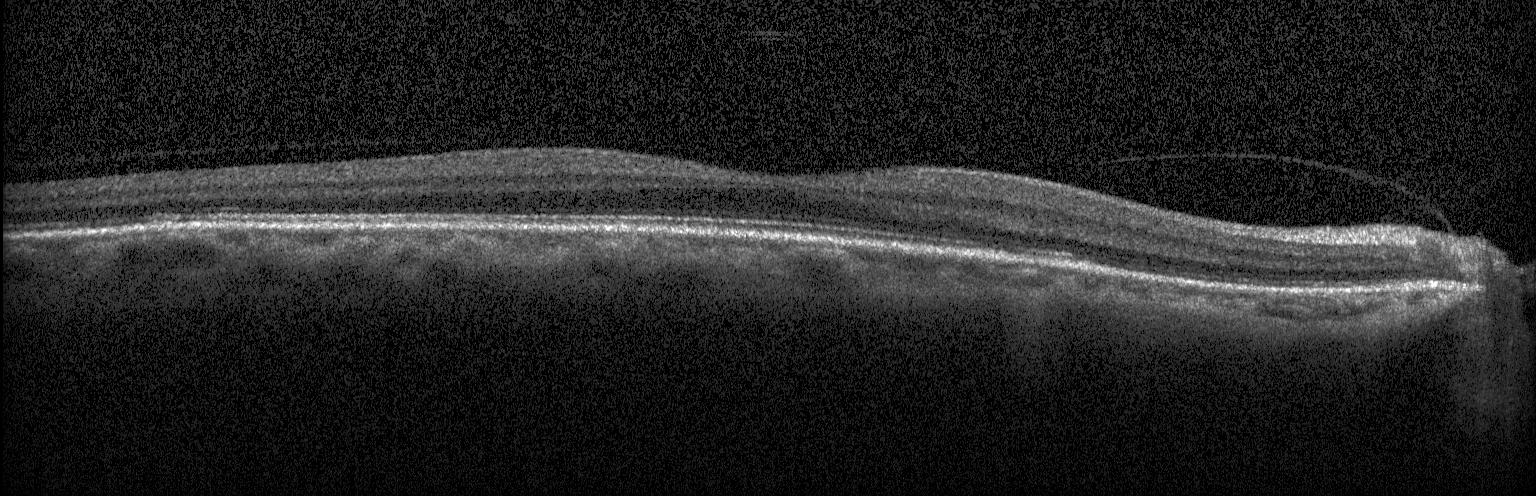 Retinal OCT cross-section showing neither choroidal neovascularization, diabetic macular edema, nor drusen.